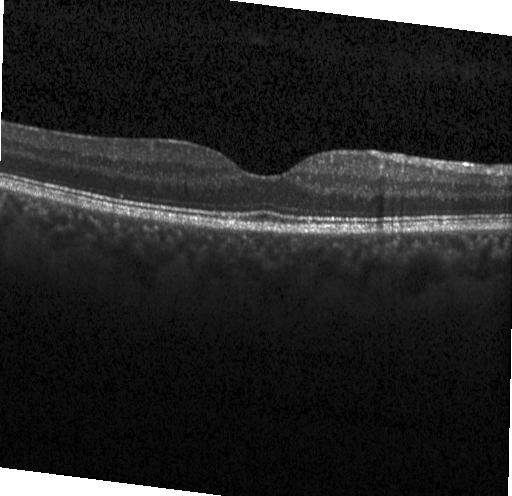 SD-OCT. OCT B-scan — The scan shows no evidence of choroidal neovascularization, diabetic macular edema, or drusen.